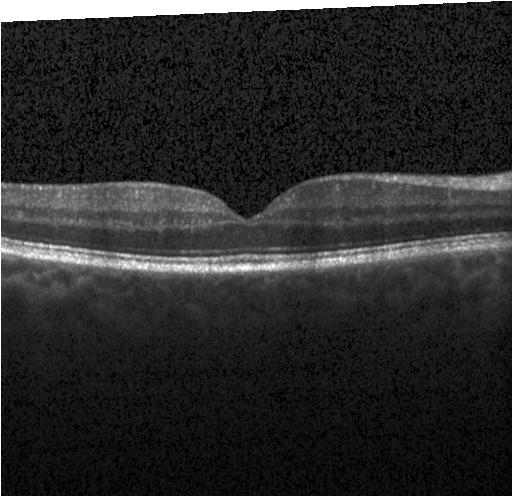 Fovea-centered. OCT line scan. Acquired on a Heidelberg Spectralis
Diagnosis: neither choroidal neovascularization, diabetic macular edema, nor drusen.